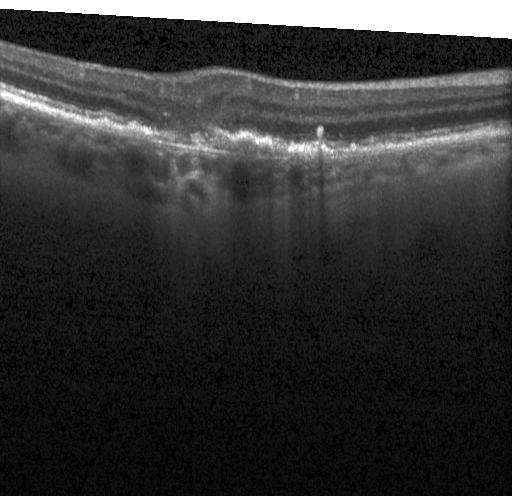

SD-OCT. Optical coherence tomography B-scan. Heidelberg Spectralis OCT system
Choroidal neovascularization.